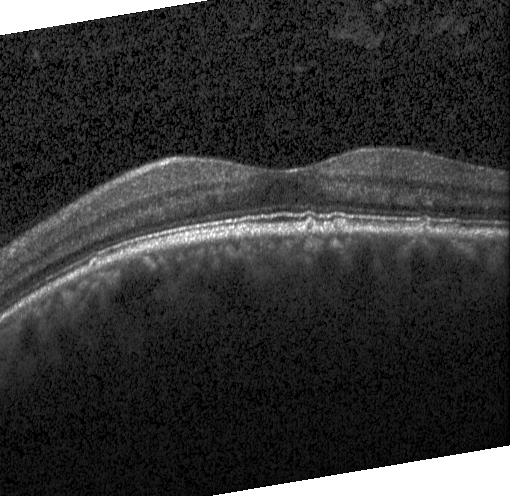 Optical coherence tomography scan
Drusen.